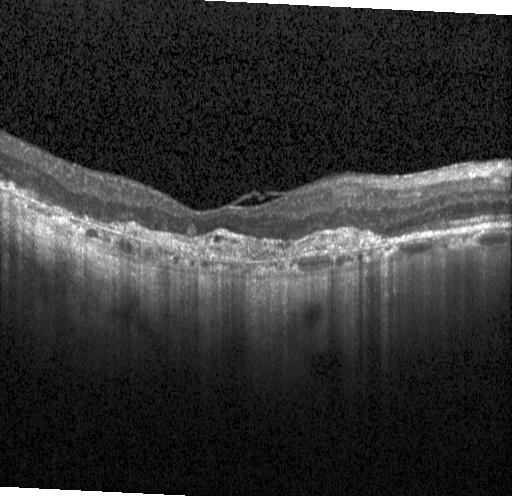

Retinal OCT B-scan, spectral-domain optical coherence tomography — Assessment: choroidal neovascularization.